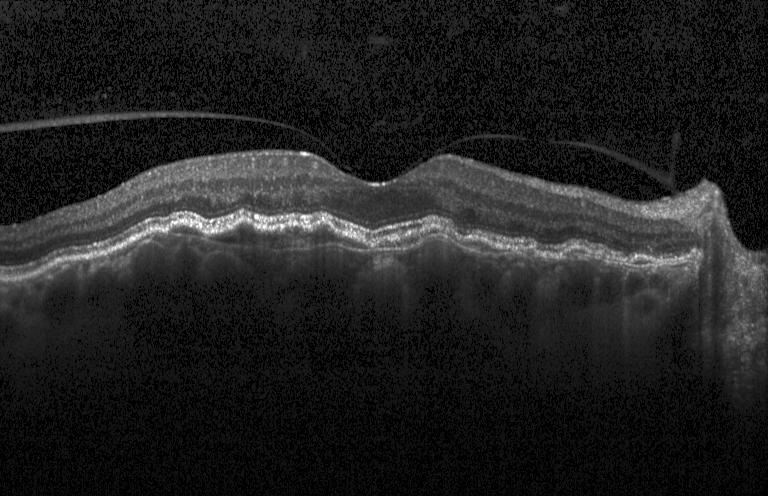
Retinal OCT cross-section.
Diagnosis: choroidal neovascularization.